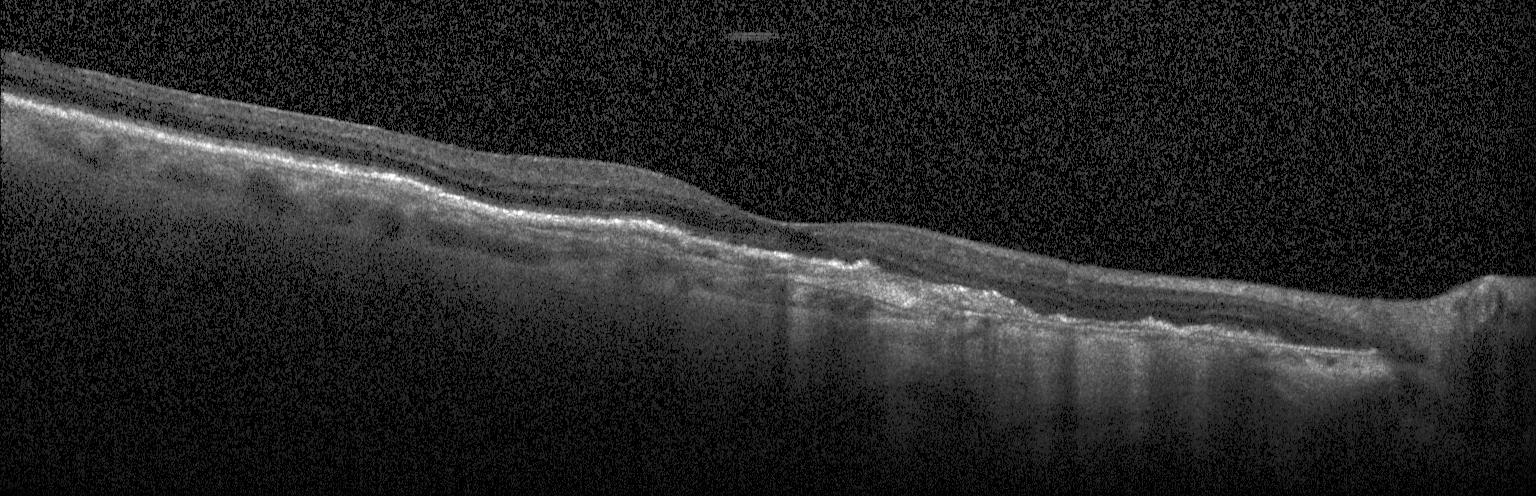

Heidelberg Spectralis, retinal OCT cross-section, SD-OCT — Impression: a choroidal neovascular membrane.